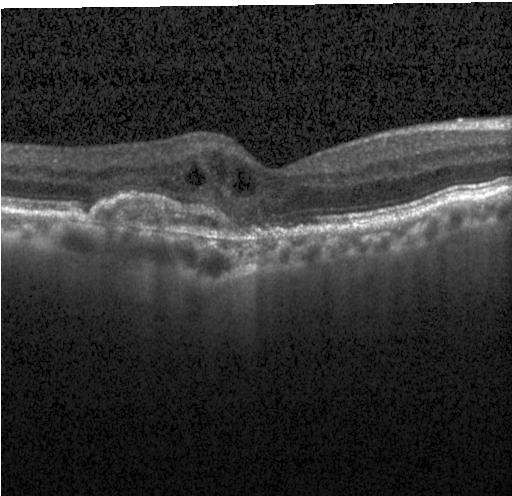 Diagnosis: a choroidal neovascular membrane.